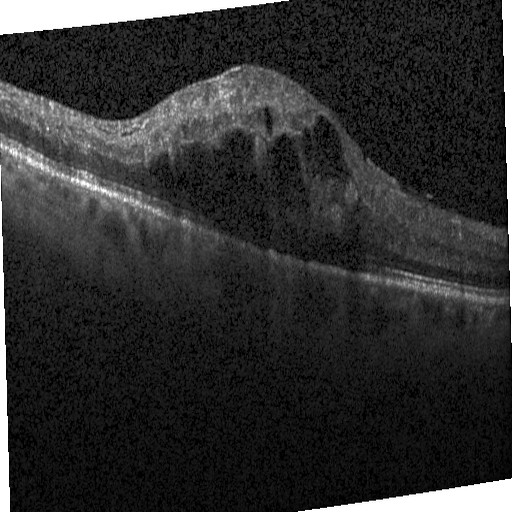 Retinal OCT cross-section — Finding: diabetic macular edema (DME).